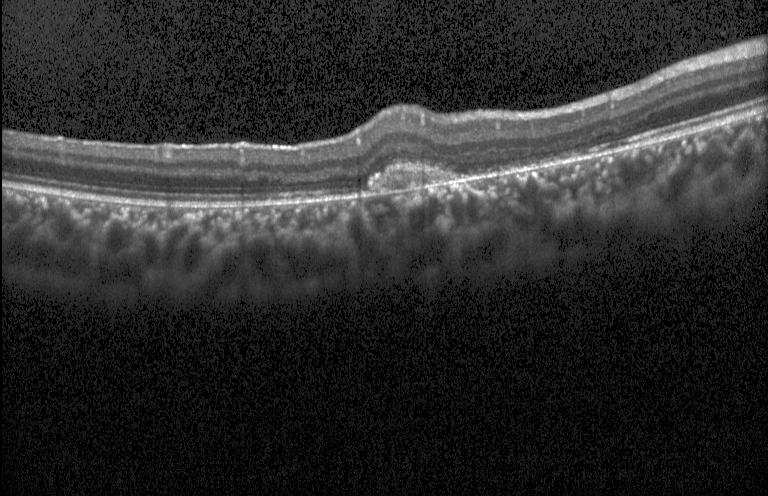
Dx: choroidal neovascularization (CNV).